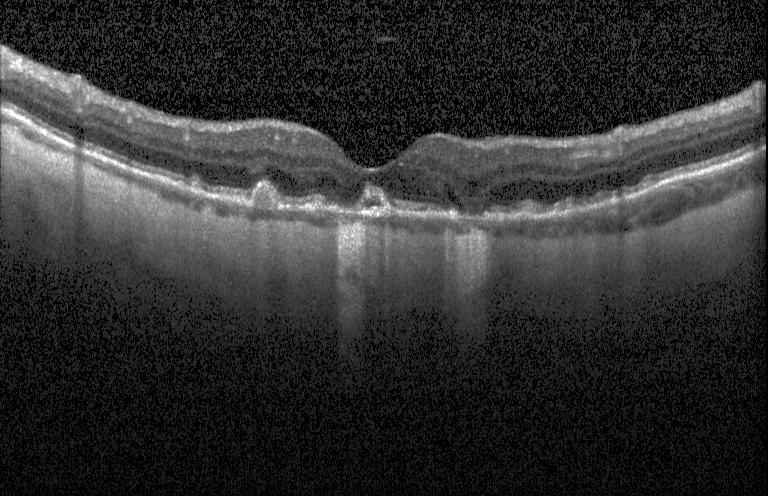

Optical coherence tomography B-scan, Heidelberg Spectralis, macular scan
Choroidal neovascularization (CNV).